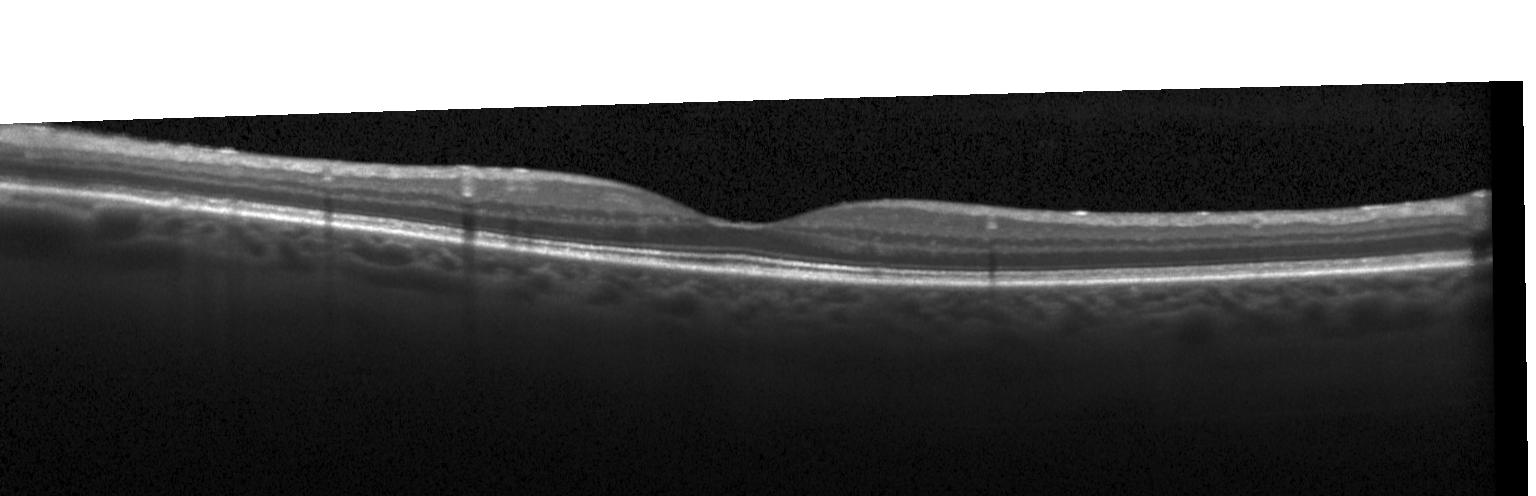

Centered on the fovea. Spectral-domain OCT. Heidelberg Spectralis. OCT line scan — Diagnosis: no choroidal neovascularization, diabetic macular edema, or drusen.